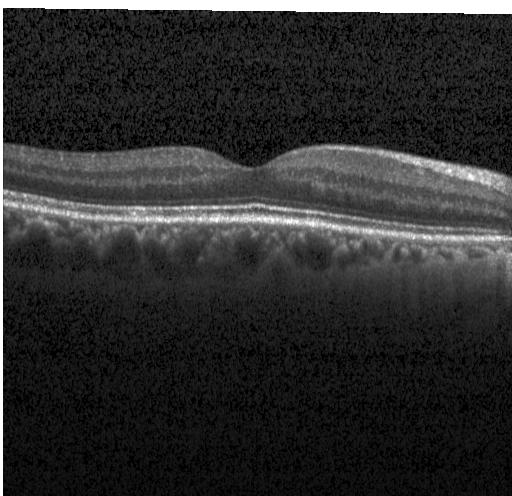 OCT B-scan, Heidelberg Spectralis OCT system, spectral-domain OCT — The scan shows no choroidal neovascularization, diabetic macular edema, or drusen.